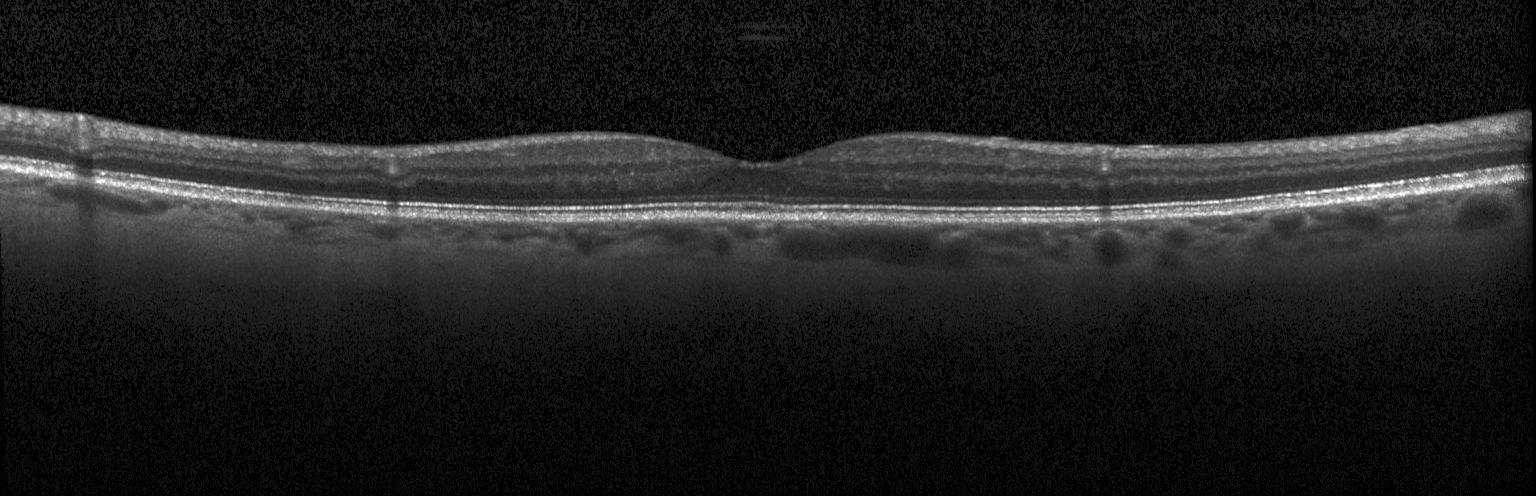
OCT B-scan, SD-OCT
Diagnosis: neither choroidal neovascularization, diabetic macular edema, nor drusen.